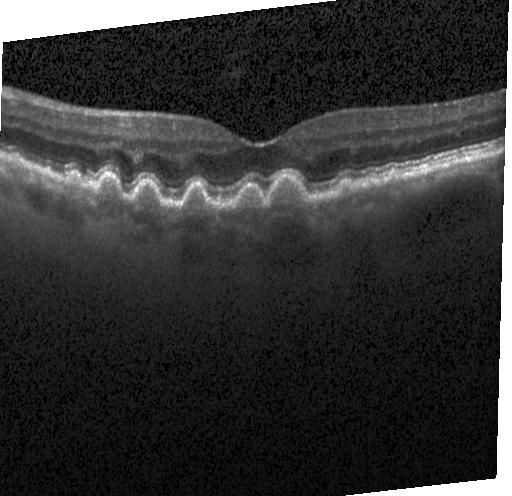 Impression: drusen.